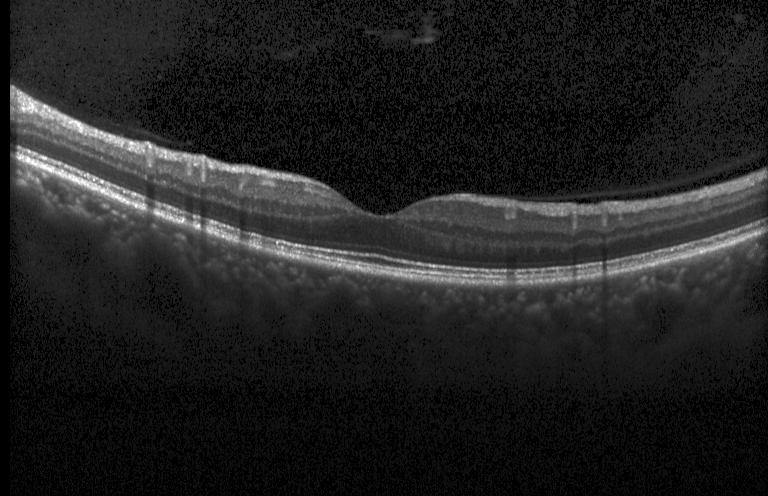 Diagnosis: no choroidal neovascularization, diabetic macular edema, or drusen.